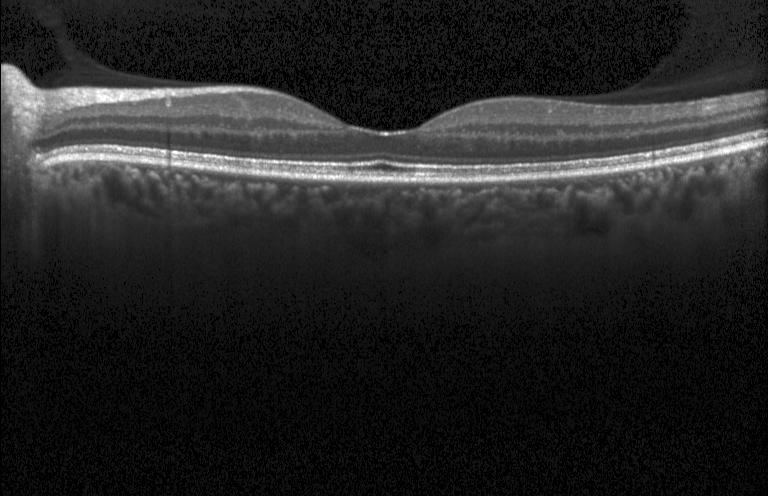 No CNV, no DME, and no drusen.